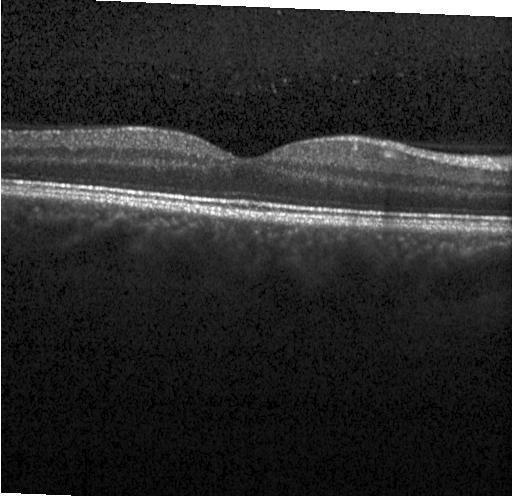 Diagnosis: no evidence of choroidal neovascularization, diabetic macular edema, or drusen.